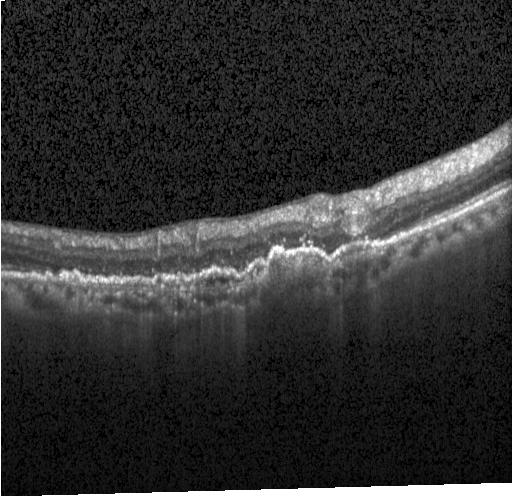

Assessment: a choroidal neovascular membrane.